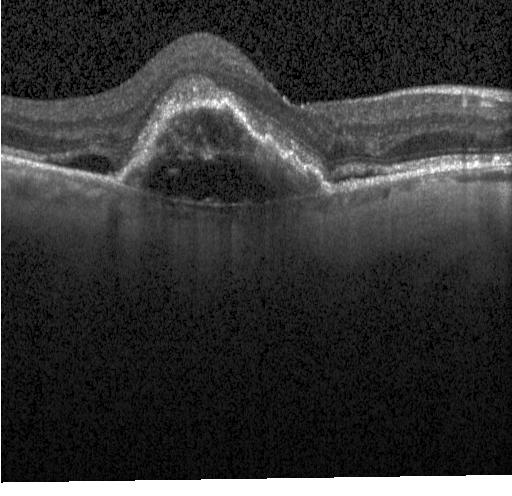 Assessment: a choroidal neovascular membrane.